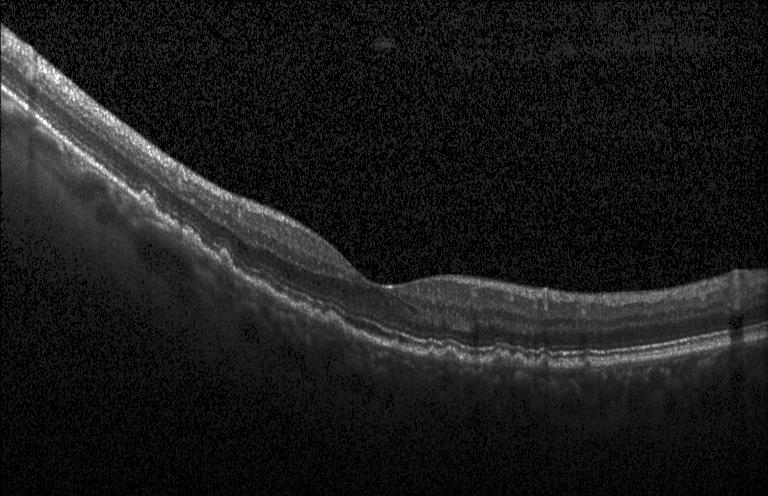

Heidelberg Spectralis; horizontal scan through the fovea; OCT line scan — Drusen.